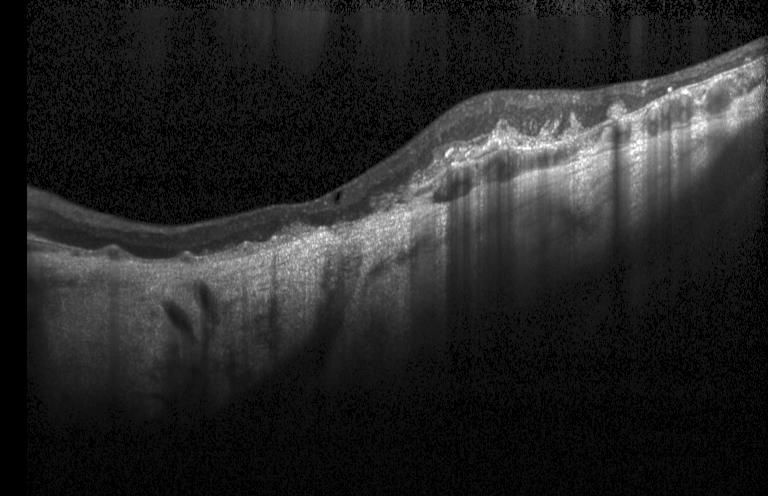

Retinal OCT B-scan — The scan shows choroidal neovascularization (CNV).